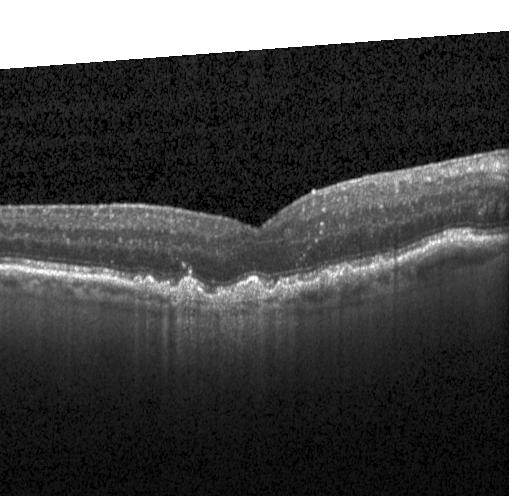
Optical coherence tomography scan — Macular OCT: choroidal neovascularization.